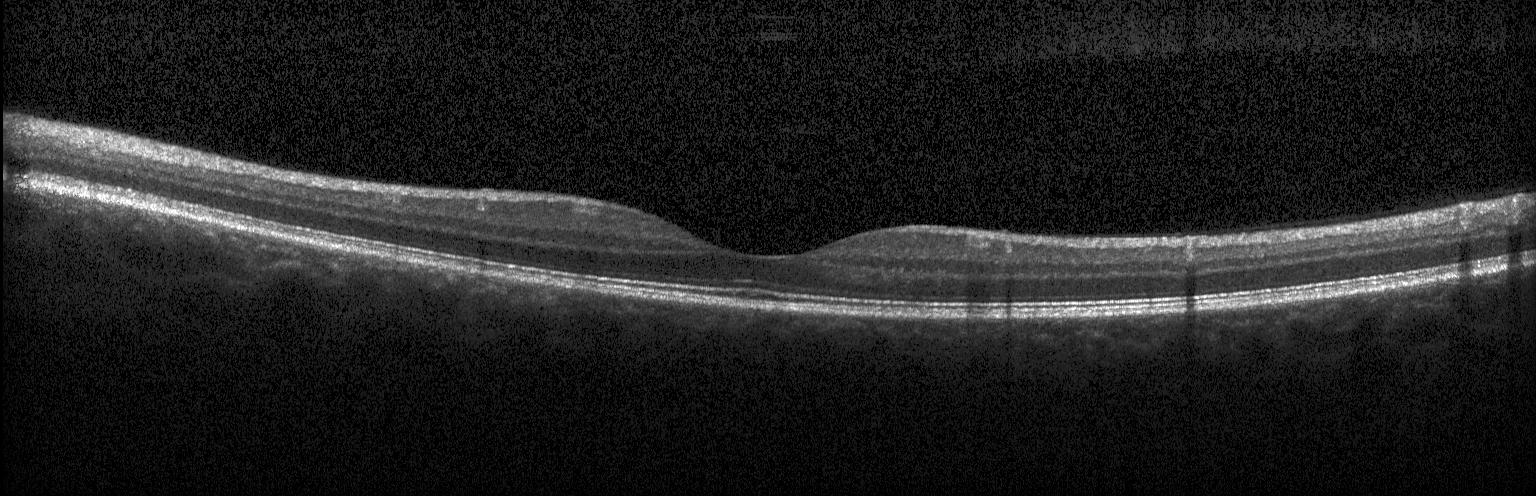
Macular OCT: no choroidal neovascularization, no diabetic macular edema, and no drusen.